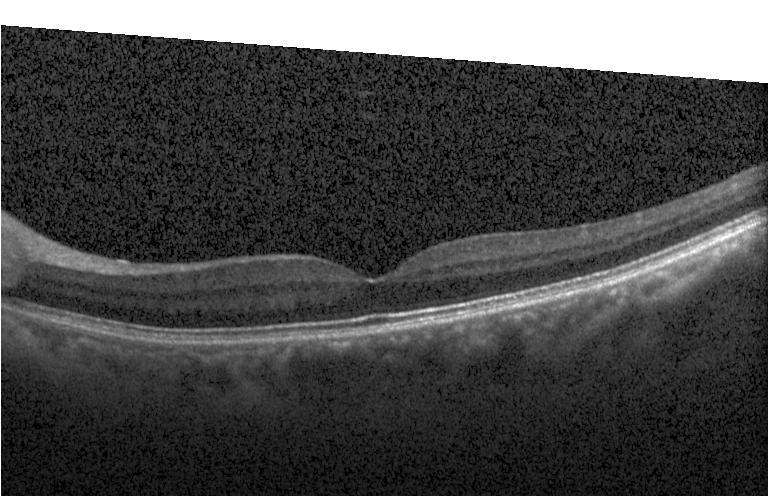
Impression: neither CNV, DME, nor drusen.